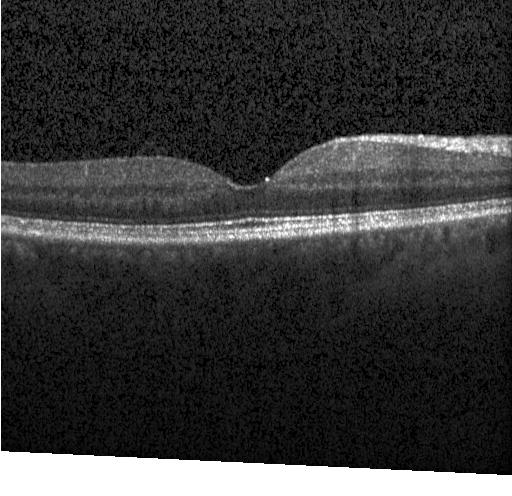
SD-OCT; OCT line scan; macular scan. This B-scan demonstrates no choroidal neovascularization, diabetic macular edema, or drusen.